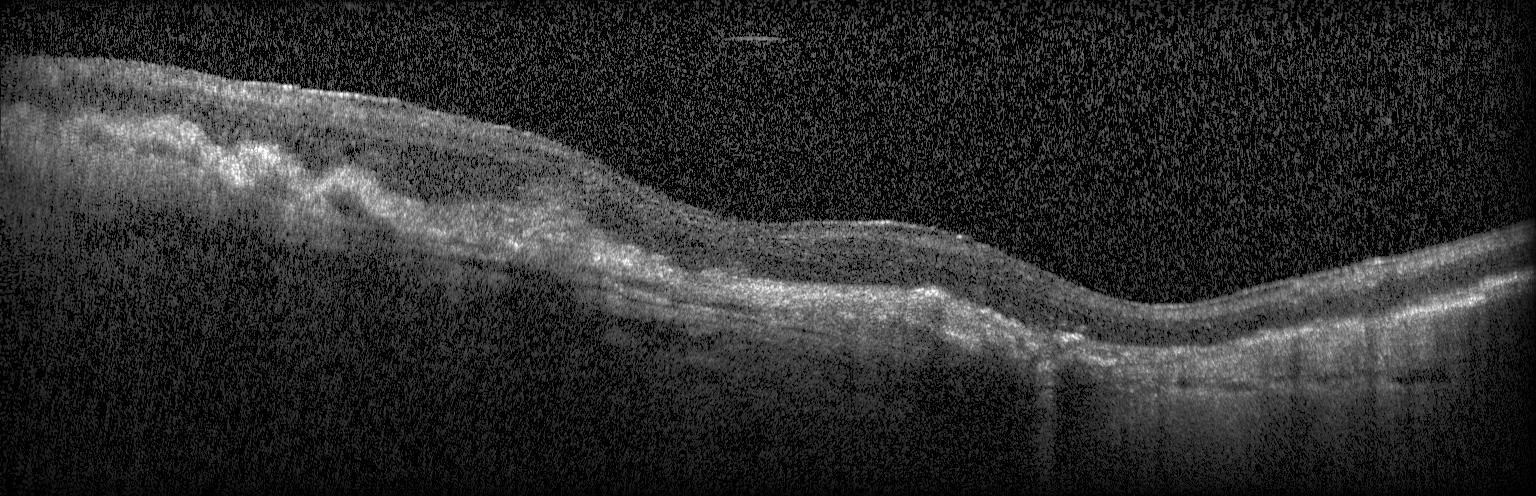 OCT B-scan
This B-scan demonstrates a choroidal neovascular membrane.